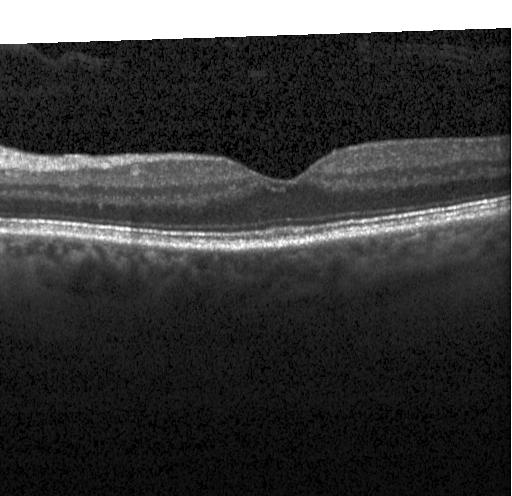 Spectral-domain OCT B-scan: neither choroidal neovascularization, diabetic macular edema, nor drusen.